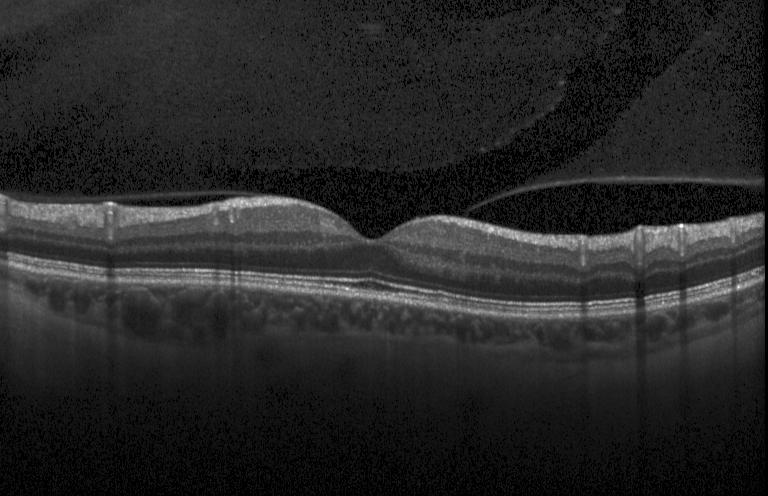 Spectral-domain OCT B-scan: neither choroidal neovascularization, diabetic macular edema, nor drusen.